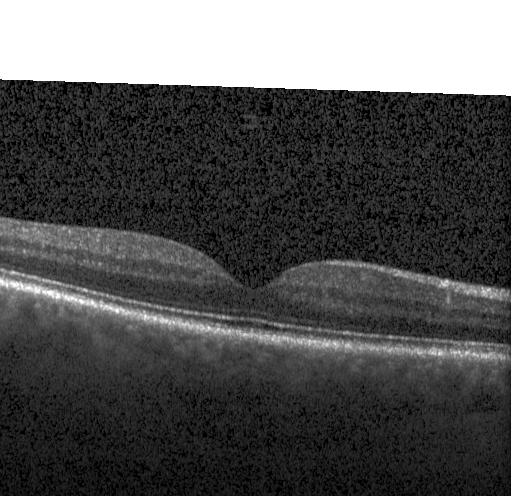
Optical coherence tomography scan
This B-scan demonstrates neither CNV, DME, nor drusen.